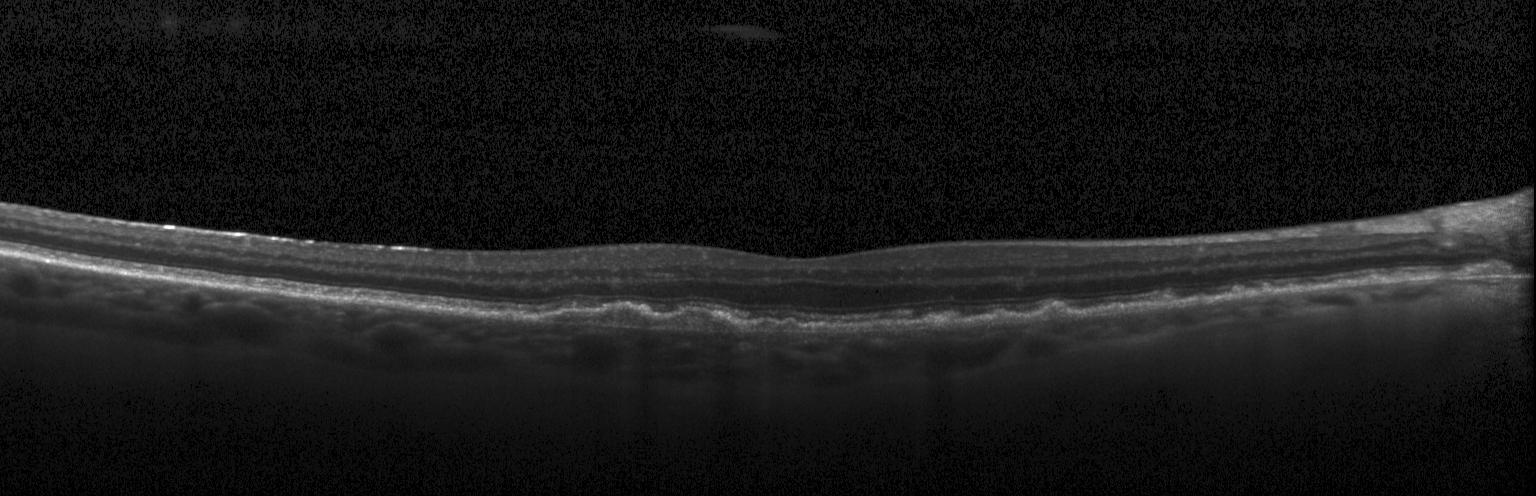

Retinal OCT cross-section showing choroidal neovascularization (CNV).